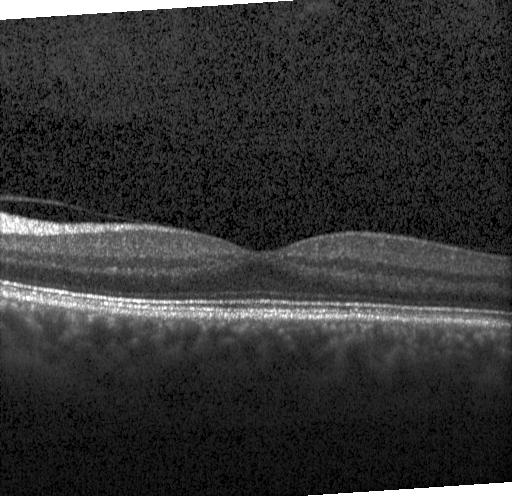

OCT line scan. Dx: no evidence of choroidal neovascularization, diabetic macular edema, or drusen.